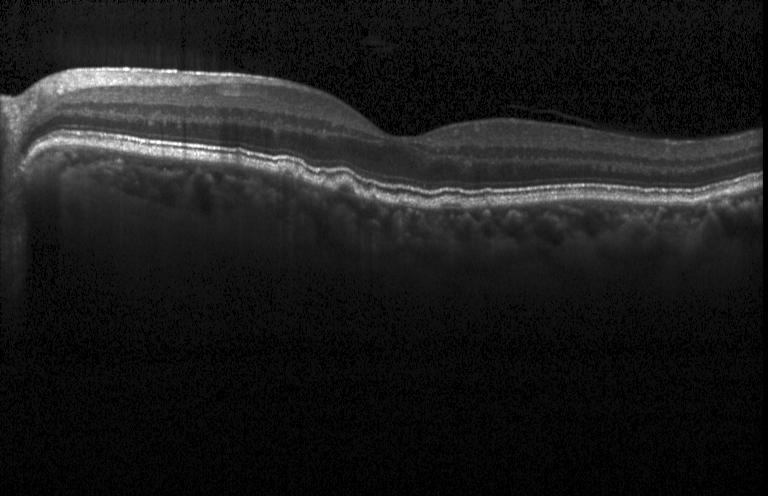

Dx: sub-RPE drusenoid deposits.